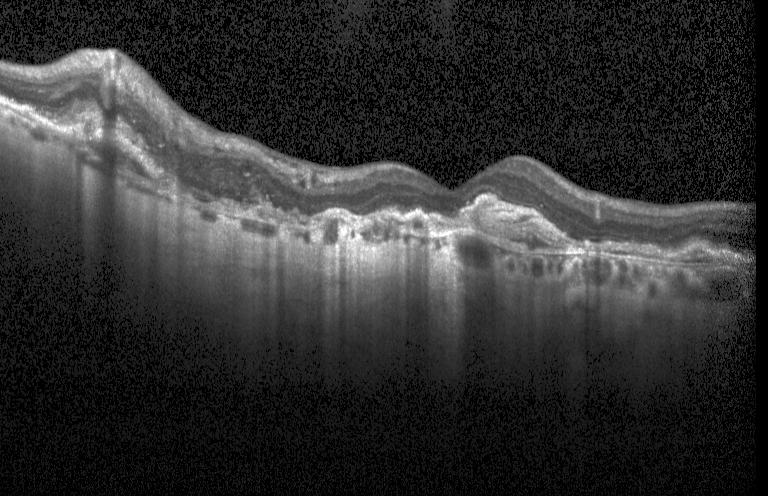

OCT B-scan · Heidelberg Spectralis · through the macula. This B-scan demonstrates choroidal neovascularization (CNV).